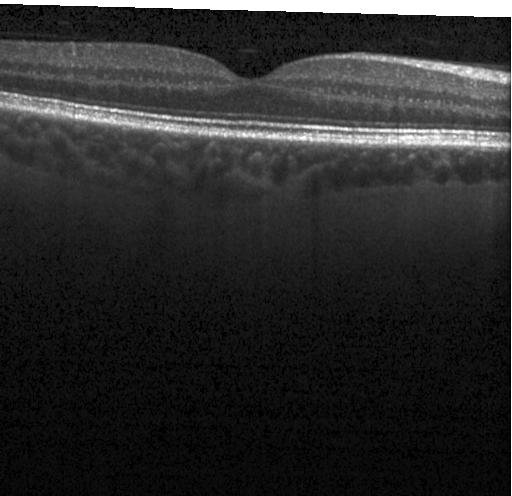 Retinal OCT B-scan.
Finding: no CNV, no DME, and no drusen.